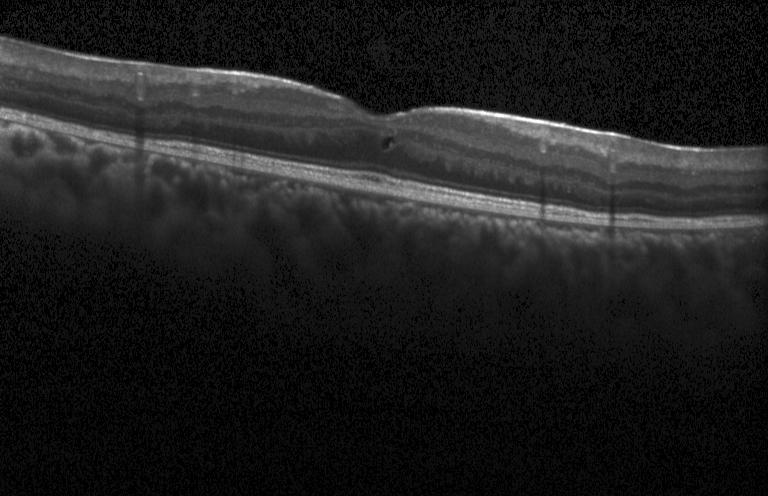

Spectral-domain OCT, through the macula, OCT line scan
Dx: DME.